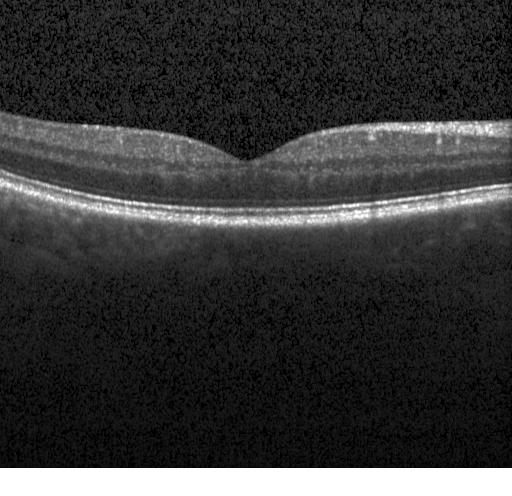 Diagnosis: no choroidal neovascularization, no diabetic macular edema, and no drusen.